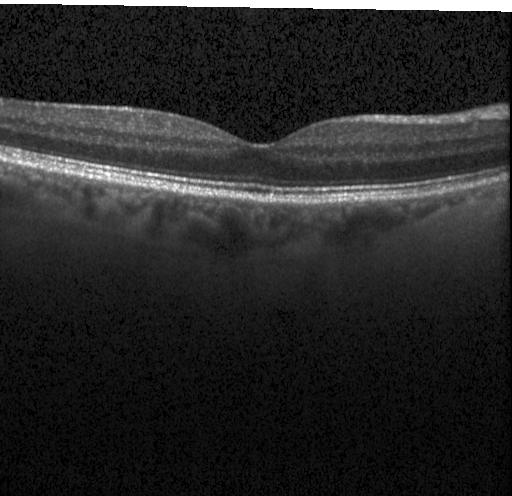

OCT B-scan showing no evidence of CNV, DME, or drusen.